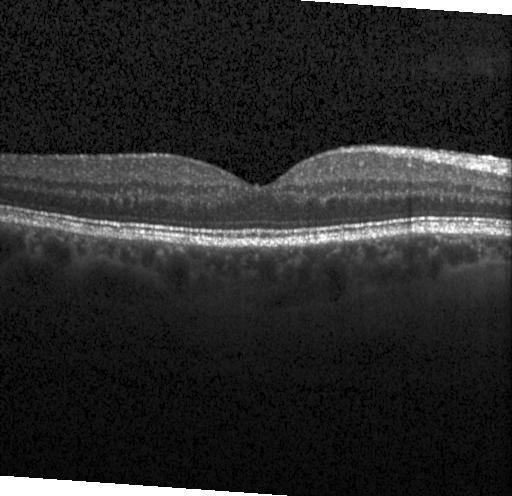 Optical coherence tomography scan; spectral-domain optical coherence tomography; instrument: Heidelberg Spectralis; macular scan. The scan shows neither choroidal neovascularization, diabetic macular edema, nor drusen.